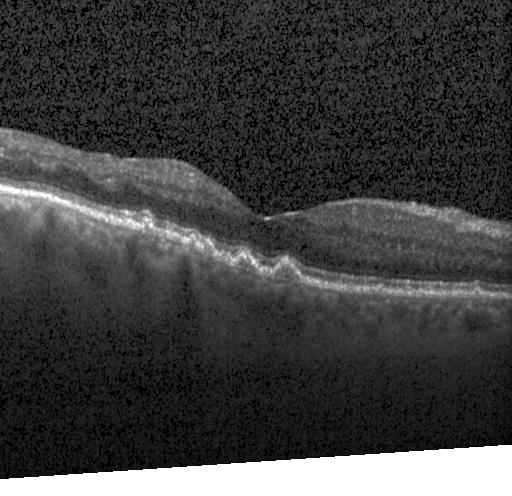 Acquired on a Heidelberg Spectralis; SD-OCT; macular scan; OCT line scan
Sub-RPE drusenoid deposits.